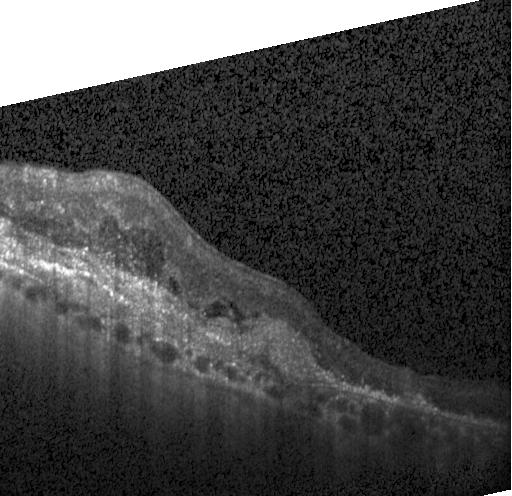 Retinal OCT cross-section. Spectral-domain OCT. Fovea-centered — Diagnosis: choroidal neovascularization (CNV).